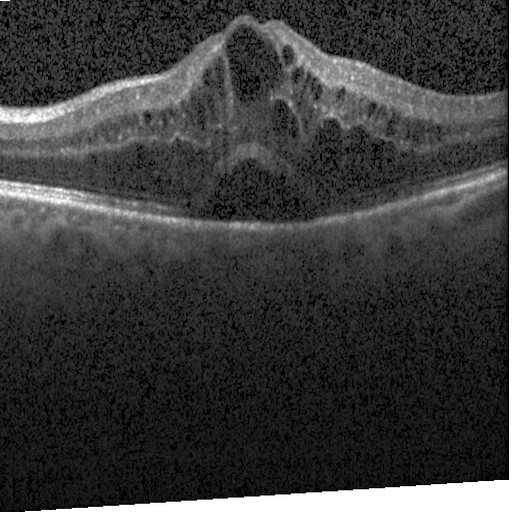 Fovea-centered; retinal OCT cross-section; SD-OCT; Heidelberg Spectralis OCT system — Finding: diabetic macular edema.